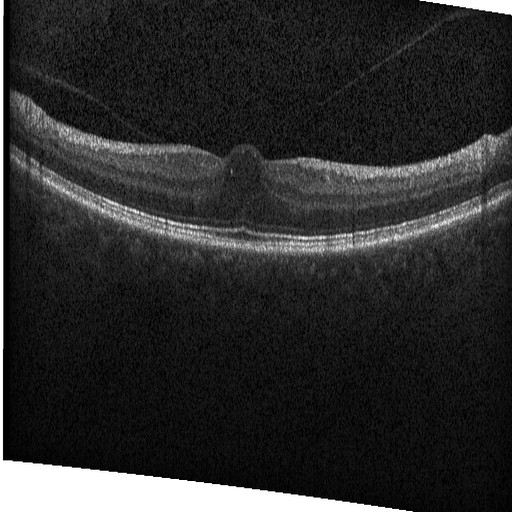

Diabetic macular edema.